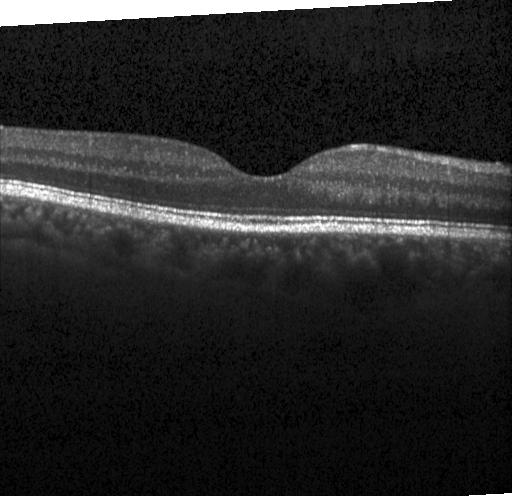 Centered on the fovea; optical coherence tomography B-scan.
Macular OCT: no choroidal neovascularization, diabetic macular edema, or drusen.